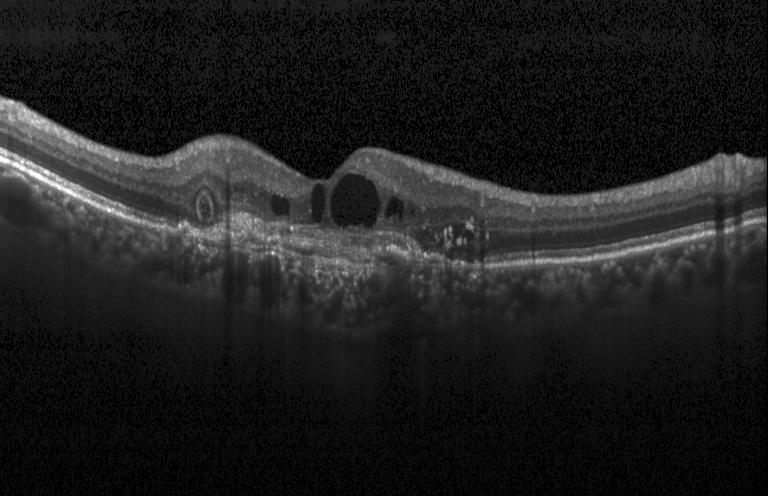

Retinal OCT B-scan, macular scan, spectral-domain optical coherence tomography, Heidelberg Spectralis OCT system
Assessment: choroidal neovascularization (CNV).